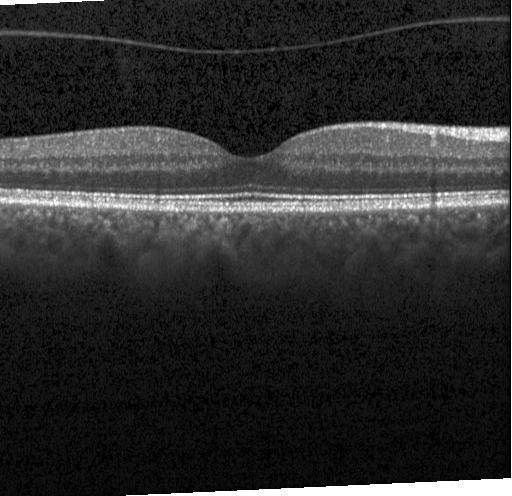
Spectral-domain optical coherence tomography. Heidelberg Spectralis. Optical coherence tomography B-scan — Dx: no evidence of CNV, DME, or drusen.